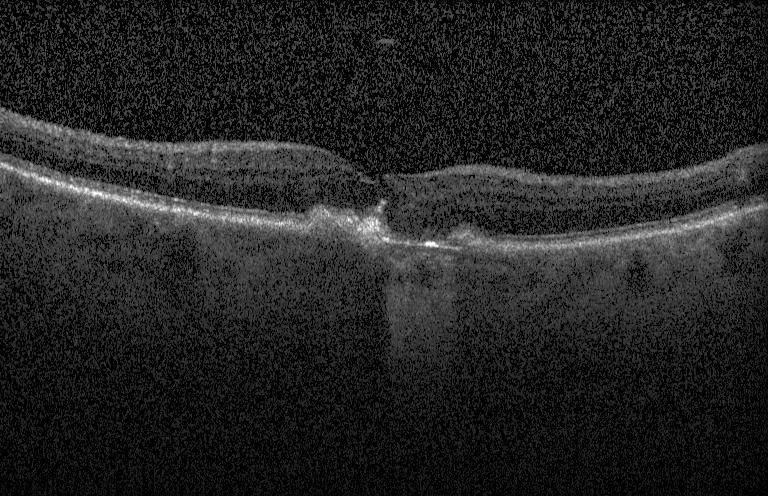

Optical coherence tomography scan. Finding: CNV.